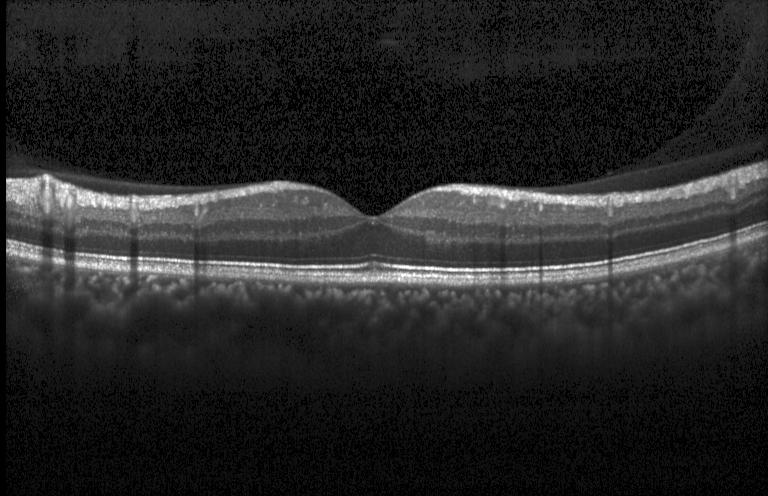

Spectral-domain OCT B-scan: neither choroidal neovascularization, diabetic macular edema, nor drusen.